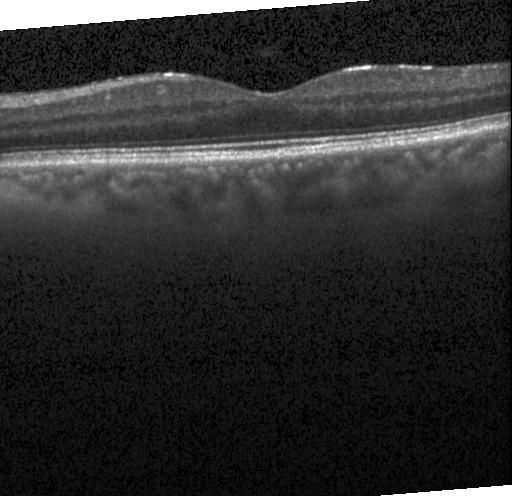

OCT B-scan showing neither choroidal neovascularization, diabetic macular edema, nor drusen.